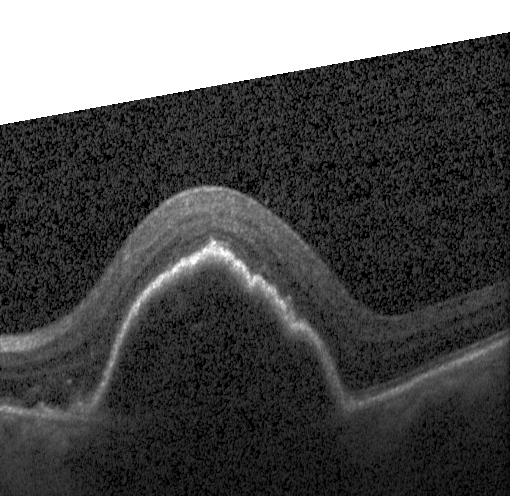
Dx: a choroidal neovascular membrane.